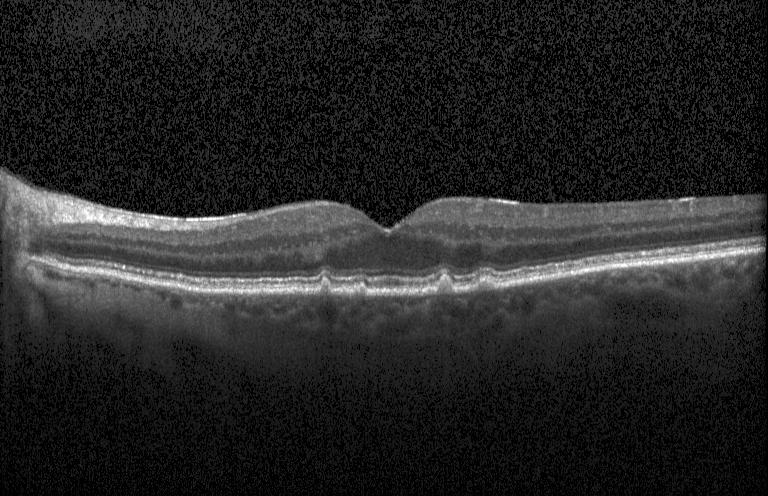
Heidelberg Spectralis OCT system, spectral-domain optical coherence tomography, retinal OCT B-scan, fovea-centered. Assessment: drusen.